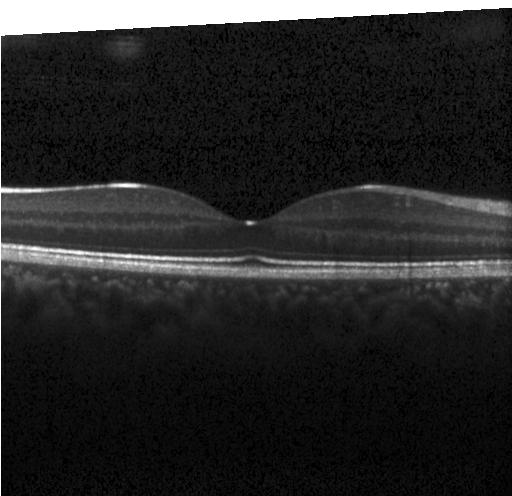 Spectral-domain optical coherence tomography, Heidelberg Spectralis OCT system, optical coherence tomography scan, macular scan.
Diagnosis: no evidence of choroidal neovascularization, diabetic macular edema, or drusen.